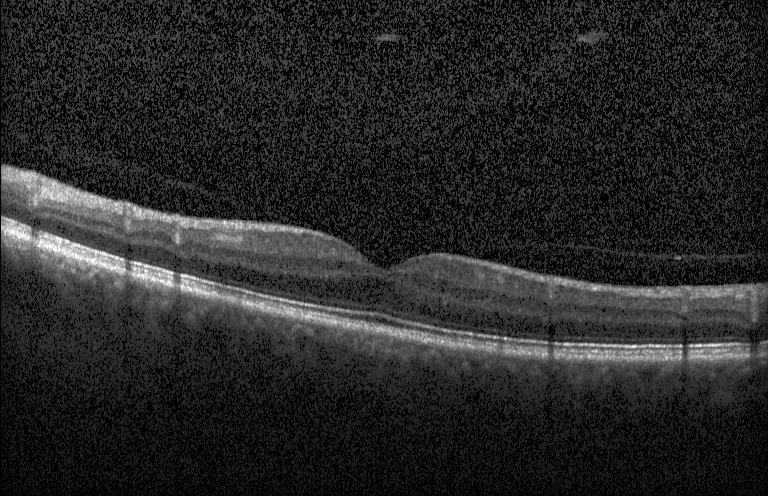 Finding: no choroidal neovascularization, no diabetic macular edema, and no drusen.